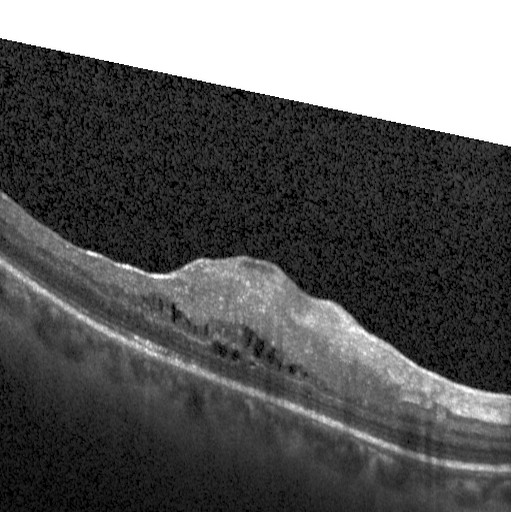

Horizontal scan through the fovea. Retinal OCT cross-section. Instrument: Heidelberg Spectralis. Finding: diabetic macular edema.